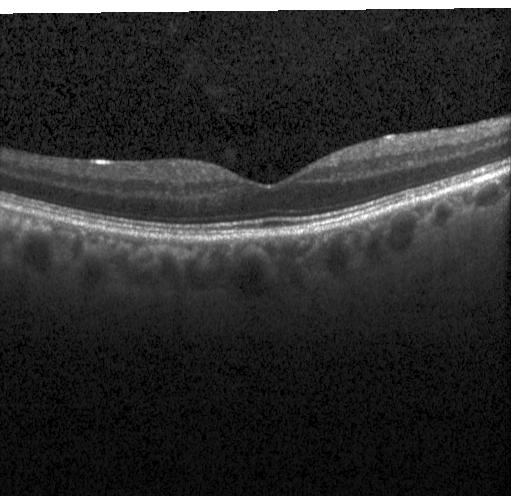

Centered on the fovea · OCT line scan.
This B-scan demonstrates no choroidal neovascularization, no diabetic macular edema, and no drusen.